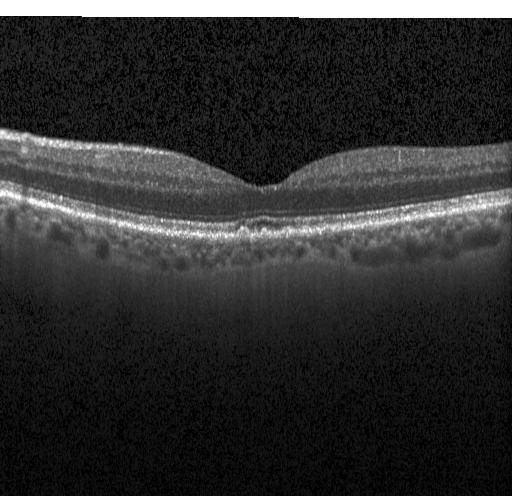

OCT line scan, Heidelberg Spectralis OCT system, spectral-domain optical coherence tomography. Diagnosis: multiple drusen.